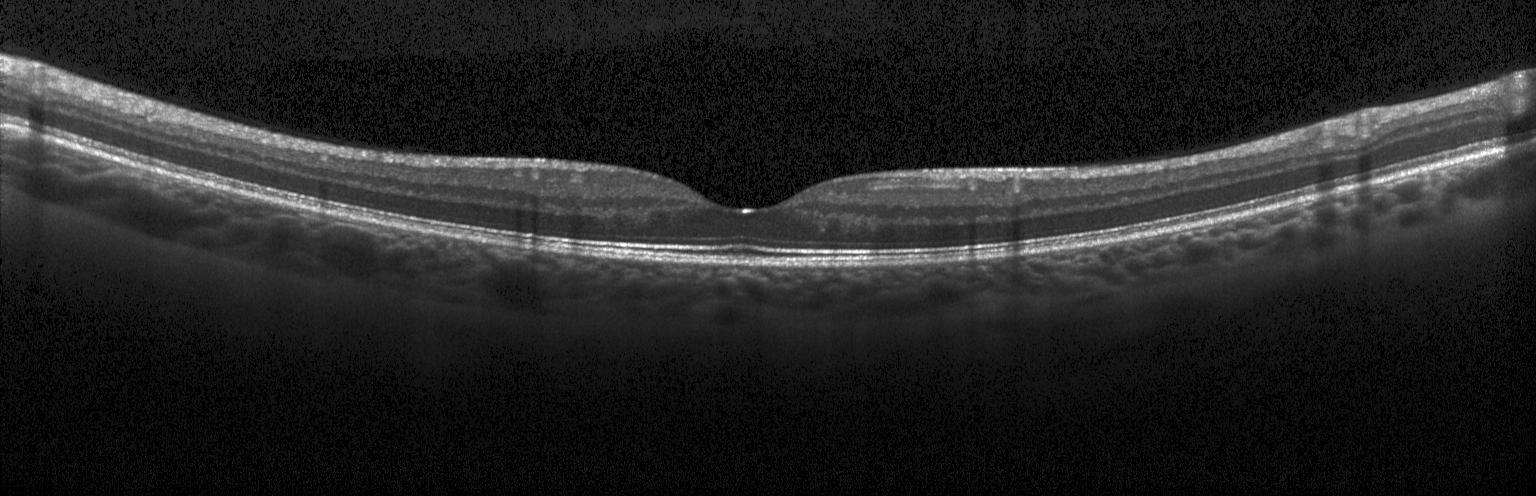 Retinal OCT B-scan, macular scan. Diagnosis: no evidence of choroidal neovascularization, diabetic macular edema, or drusen.